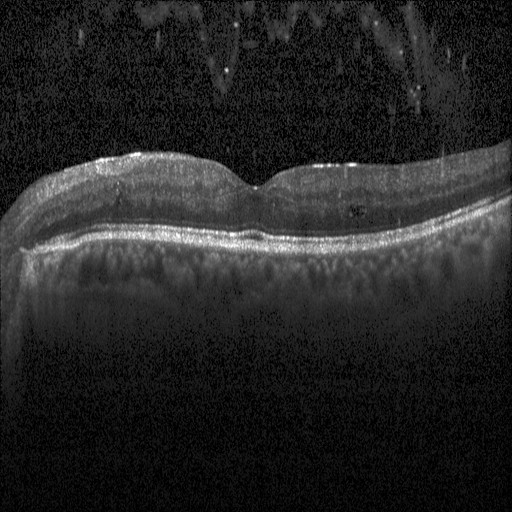
Optical coherence tomography scan. Dx: DME.